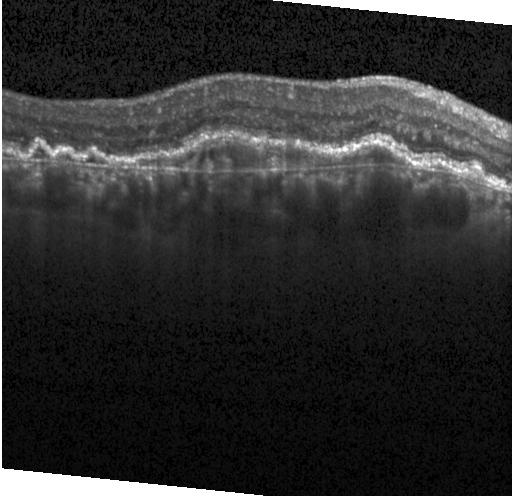 Heidelberg Spectralis OCT system. Spectral-domain optical coherence tomography. Horizontal scan through the fovea. Retinal OCT B-scan.
A choroidal neovascular membrane.